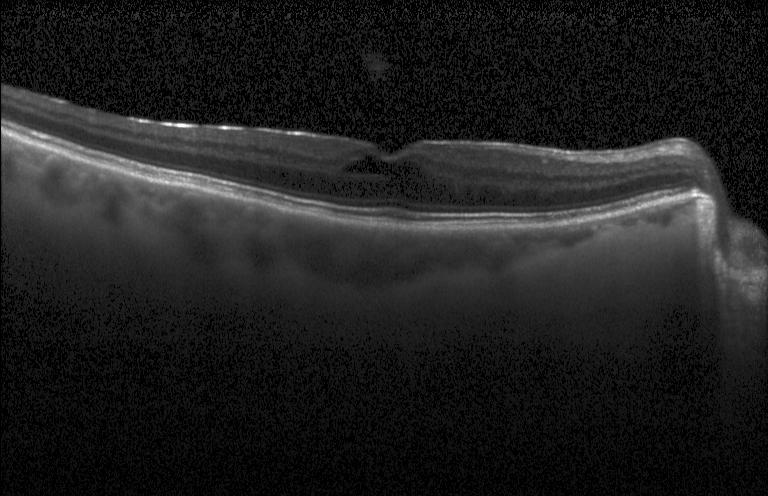

Retinal OCT cross-section showing diabetic macular edema.